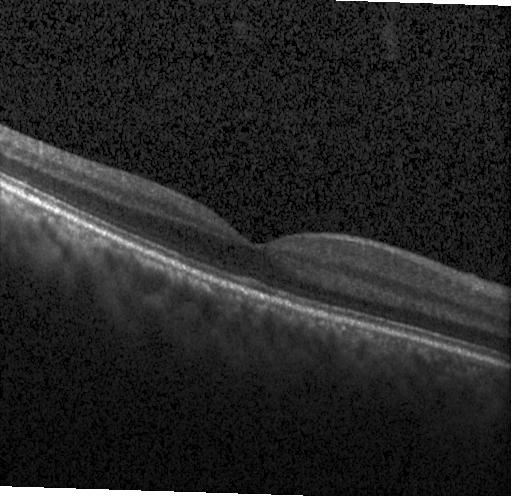 Spectral-domain optical coherence tomography, retinal OCT cross-section, macular scan. Macular OCT: no choroidal neovascularization, no diabetic macular edema, and no drusen.